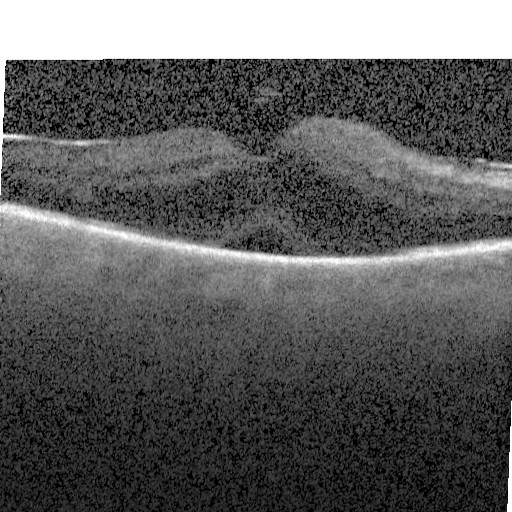 Centered on the fovea, OCT B-scan — Finding: DME.